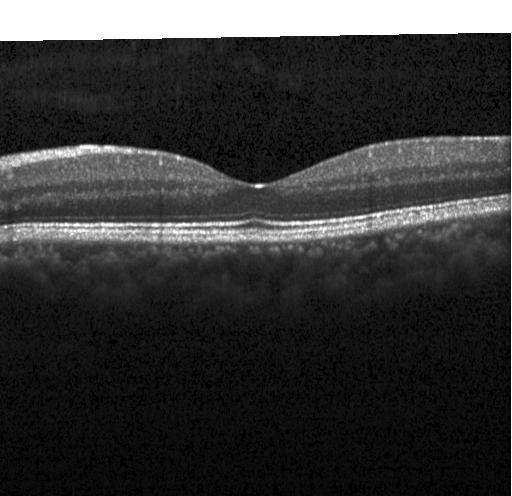 OCT line scan — OCT finding: no choroidal neovascularization, no diabetic macular edema, and no drusen.